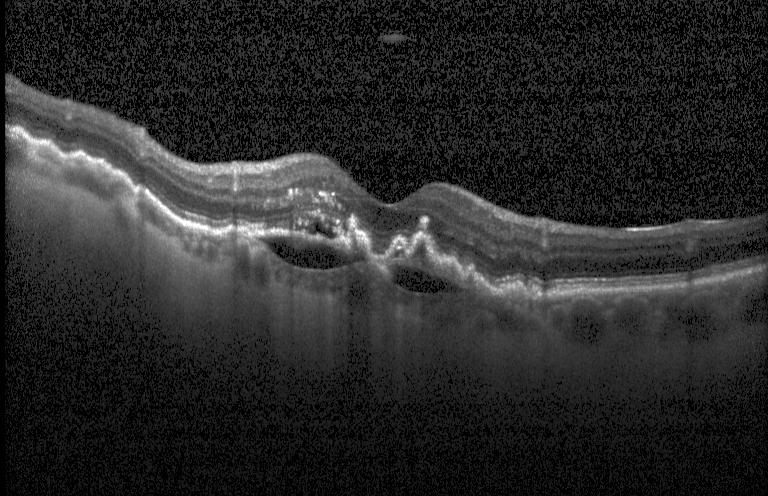
Spectral-domain optical coherence tomography, optical coherence tomography scan, fovea-centered
OCT finding: a choroidal neovascular membrane.